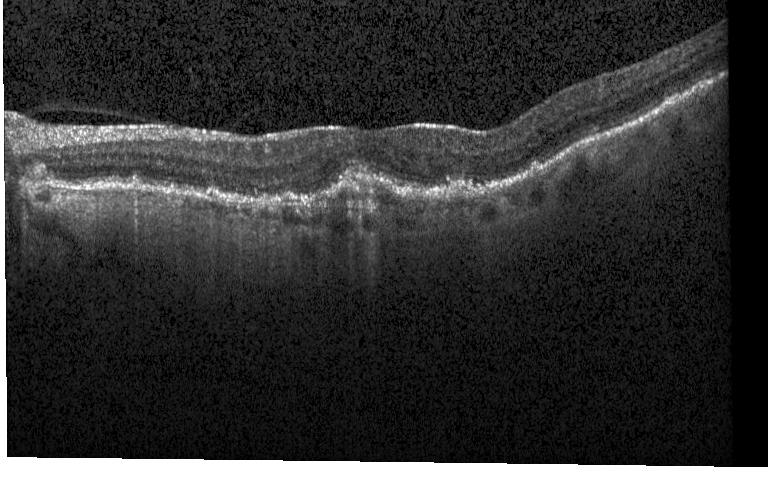 Retinal OCT B-scan
Finding: CNV.